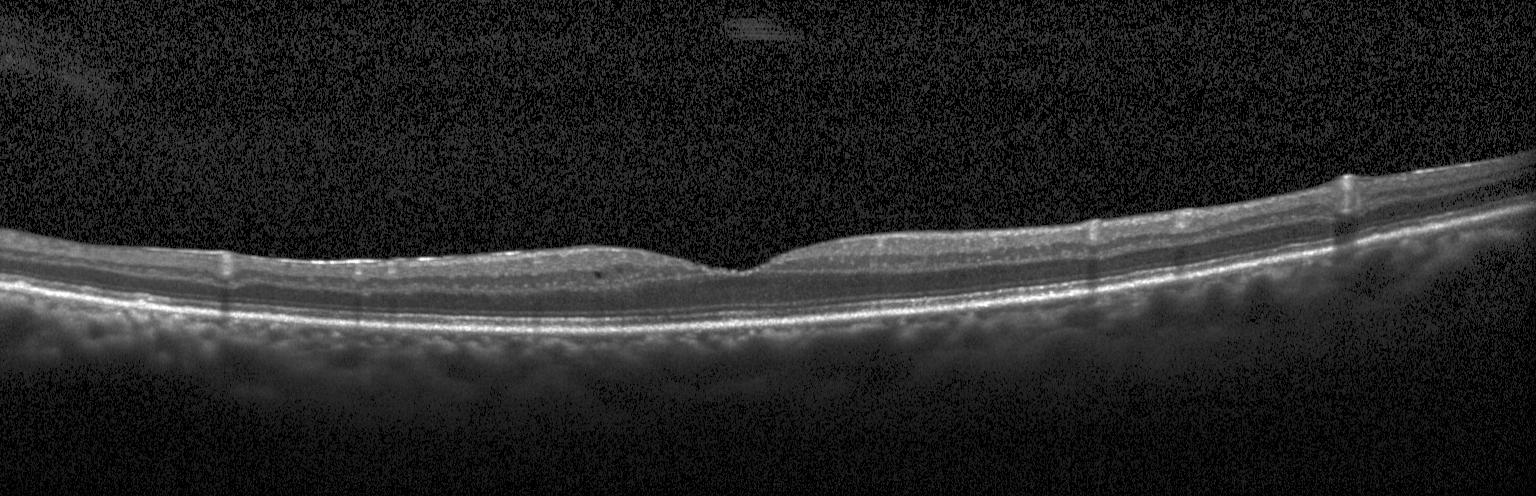 OCT finding: neither CNV, DME, nor drusen.